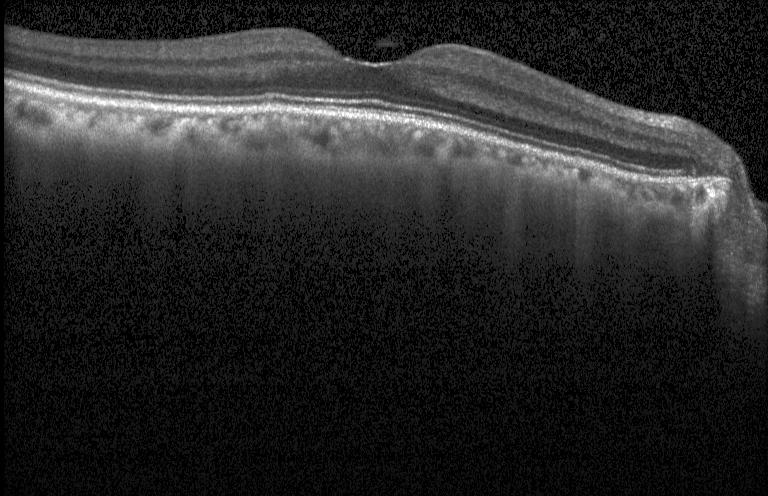
Optical coherence tomography scan; spectral-domain optical coherence tomography; Heidelberg Spectralis — OCT finding: neither choroidal neovascularization, diabetic macular edema, nor drusen.